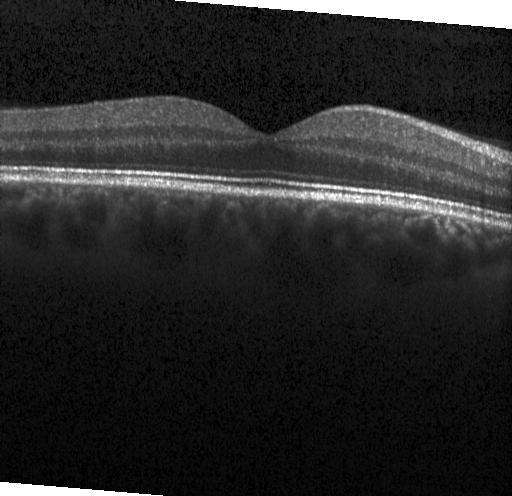

Spectral-domain OCT B-scan: no CNV, no DME, and no drusen.